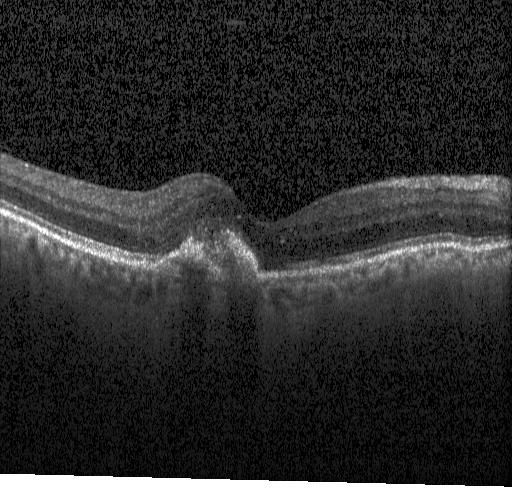 Heidelberg Spectralis. Optical coherence tomography B-scan. Macular scan. Spectral-domain optical coherence tomography. Impression: choroidal neovascularization.